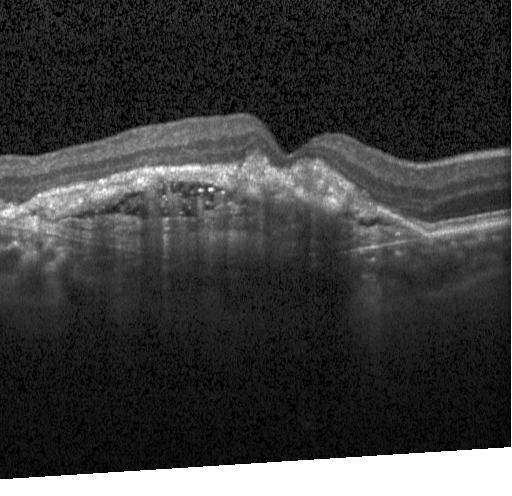

OCT B-scan; spectral-domain optical coherence tomography.
CNV.